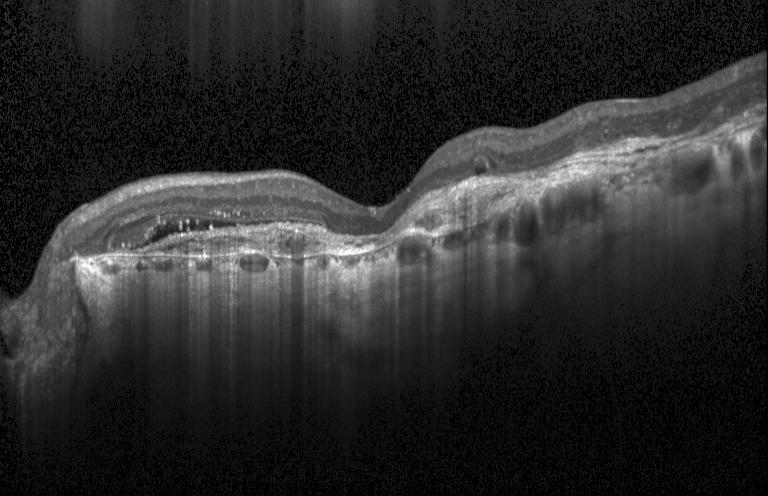
OCT line scan. Diagnosis: a choroidal neovascular membrane.